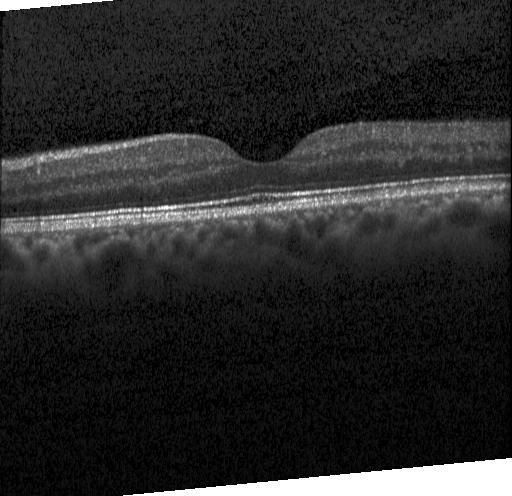

OCT line scan; acquired on a Heidelberg Spectralis; SD-OCT
Finding: no choroidal neovascularization, diabetic macular edema, or drusen.